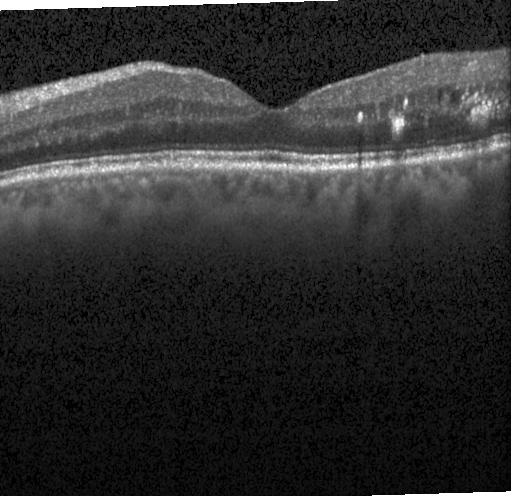 Optical coherence tomography scan, macular scan. Assessment: diabetic macular edema (DME).